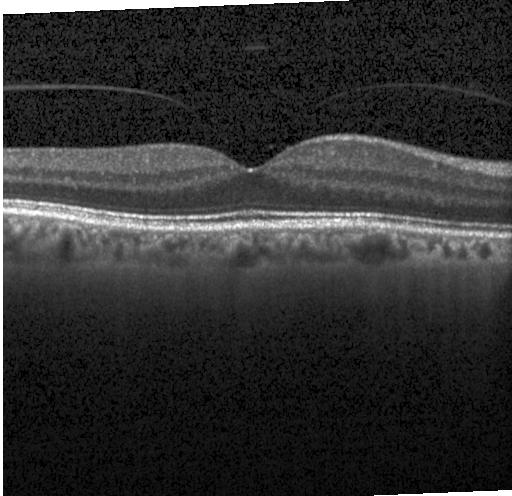
Spectral-domain OCT · acquired on a Heidelberg Spectralis · OCT line scan. Diagnosis: no choroidal neovascularization, no diabetic macular edema, and no drusen.